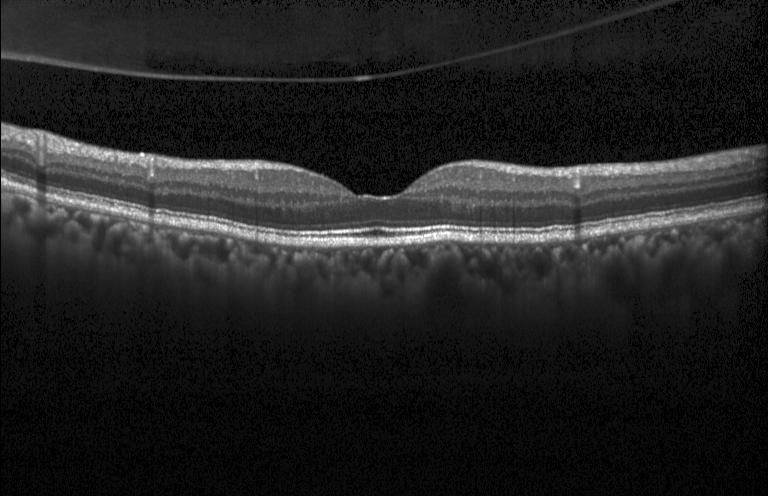
OCT line scan. Impression: no evidence of CNV, DME, or drusen.